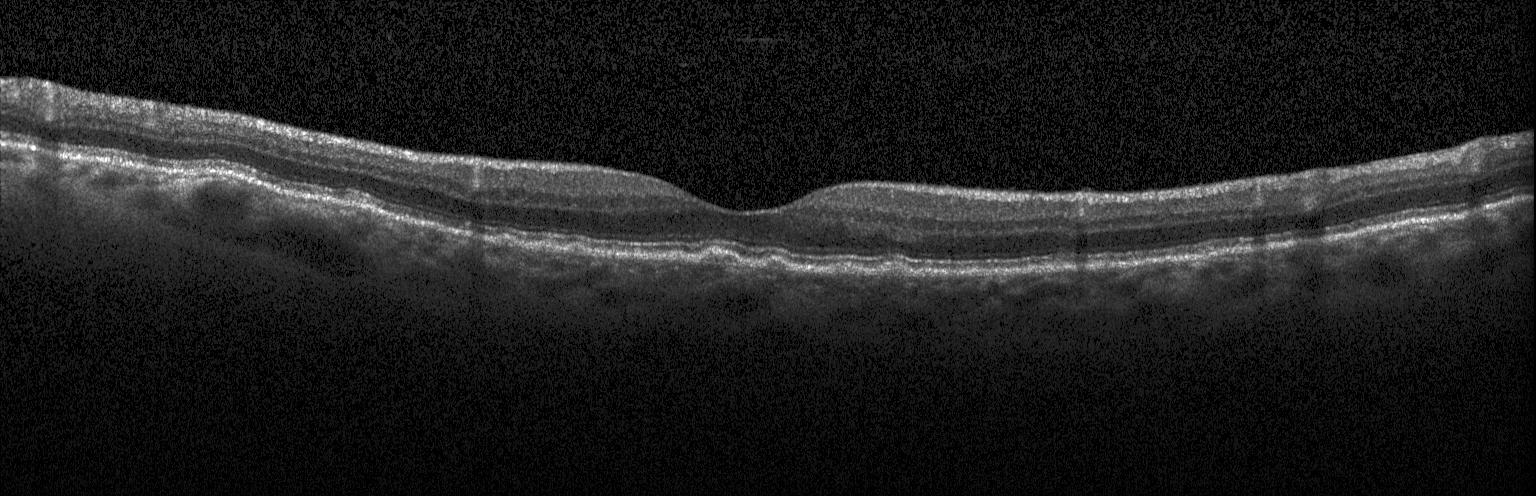

Optical coherence tomography scan.
Impression: drusen.